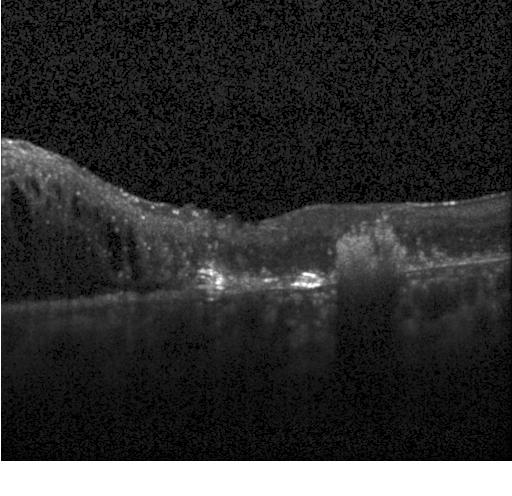

OCT line scan · macular scan
Finding: choroidal neovascularization.